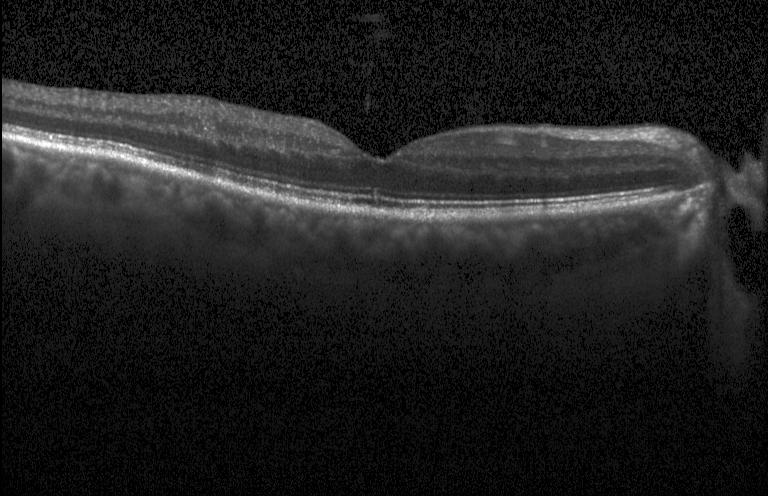 OCT scan showing no CNV, DME, or drusen.